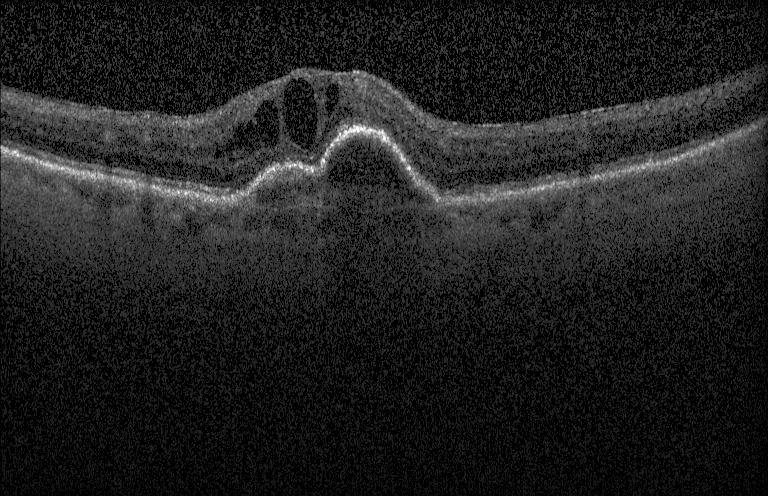

OCT line scan
Macular OCT: a choroidal neovascular membrane.